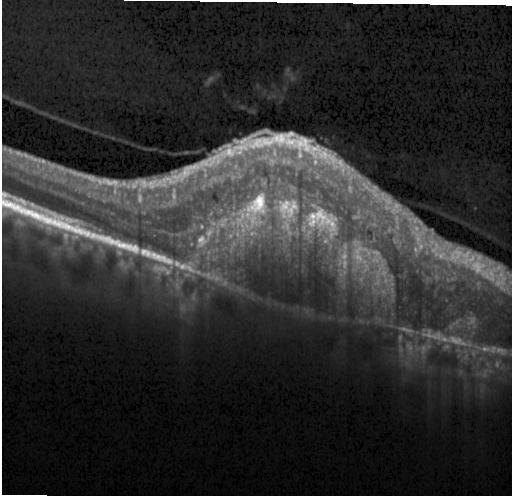

Optical coherence tomography B-scan · SD-OCT · acquired on a Heidelberg Spectralis — Finding: choroidal neovascularization.